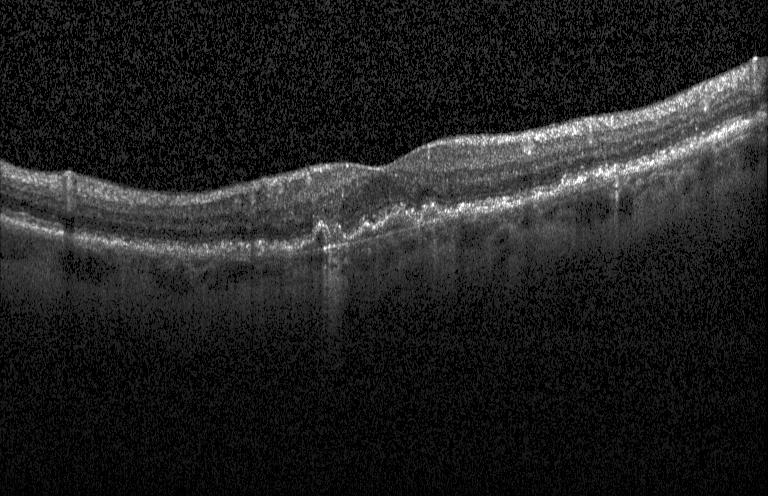

Acquired on a Heidelberg Spectralis, retinal OCT cross-section. Impression: a choroidal neovascular membrane.